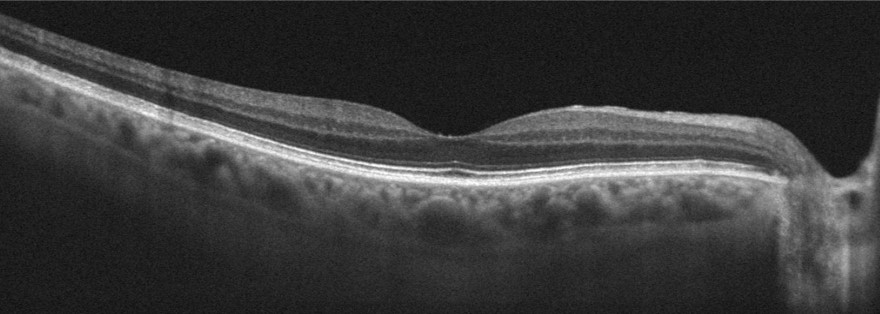 Assessment: no AMD, DME, ERM, RAO, RVO, or VID.